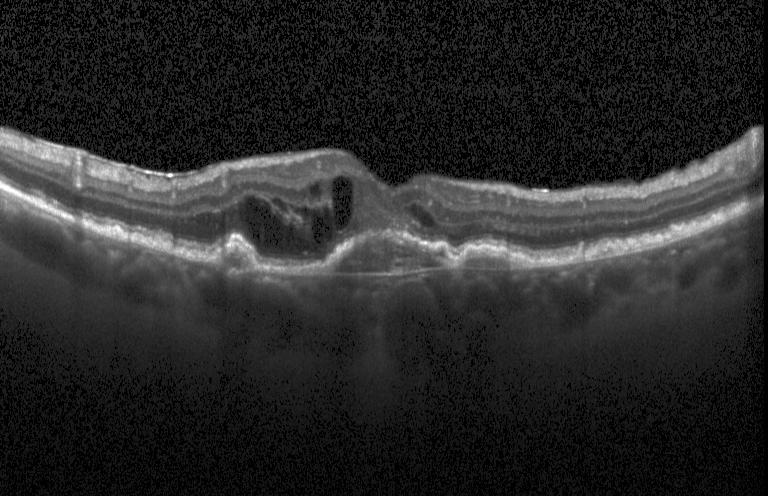

Acquired on a Heidelberg Spectralis; fovea-centered; retinal OCT B-scan — OCT finding: a choroidal neovascular membrane.